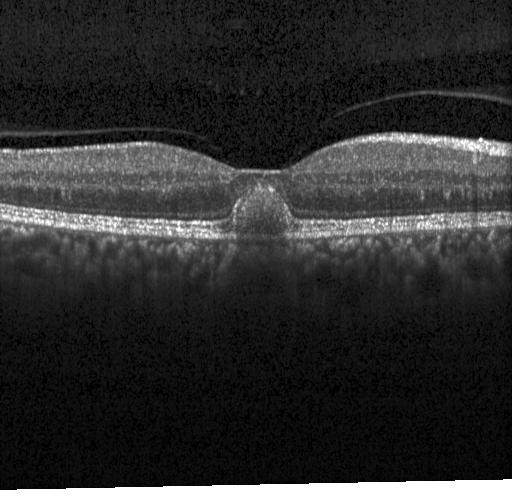

Optical coherence tomography B-scan.
Assessment: a choroidal neovascular membrane.